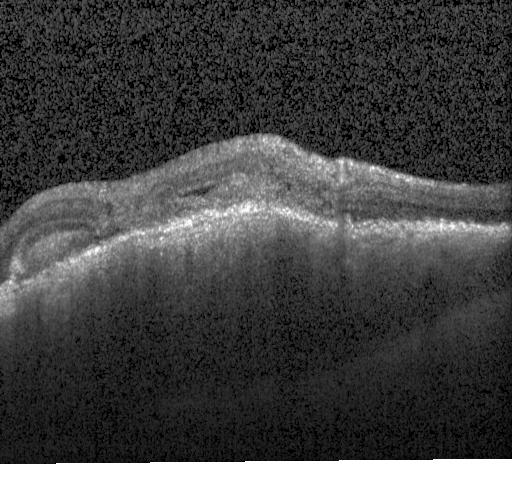 Retinal OCT cross-section — Impression: choroidal neovascularization.